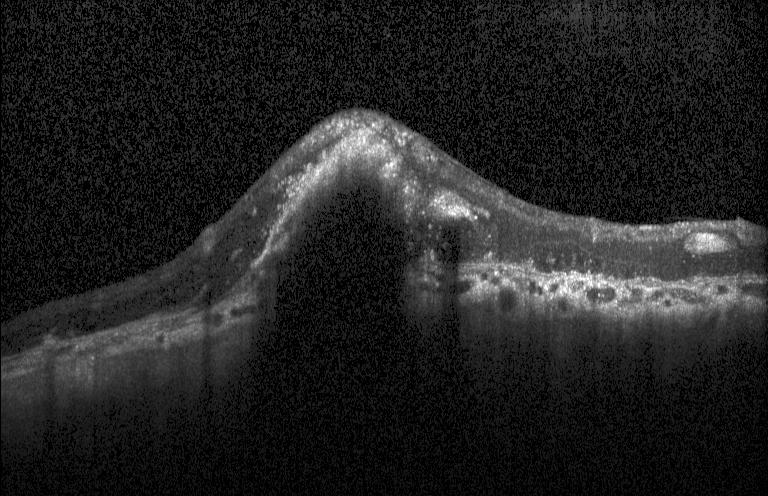

Finding: CNV.